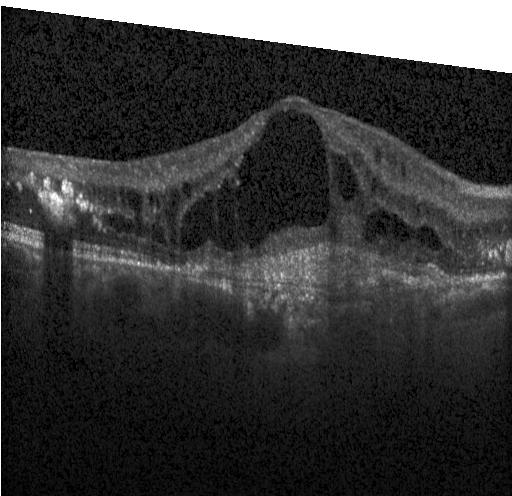

Dx: CNV.